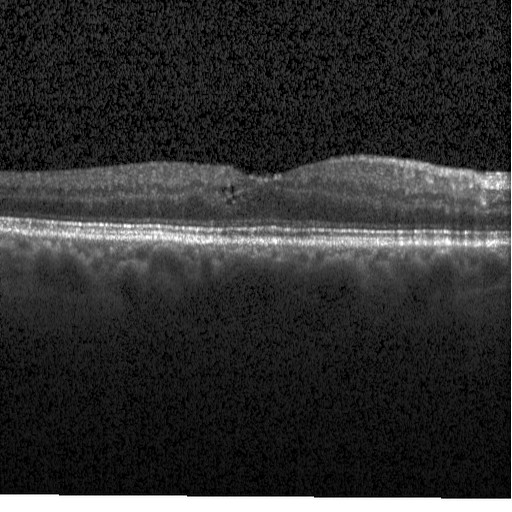

Retinal OCT B-scan · spectral-domain OCT. Finding: diabetic macular edema (DME).